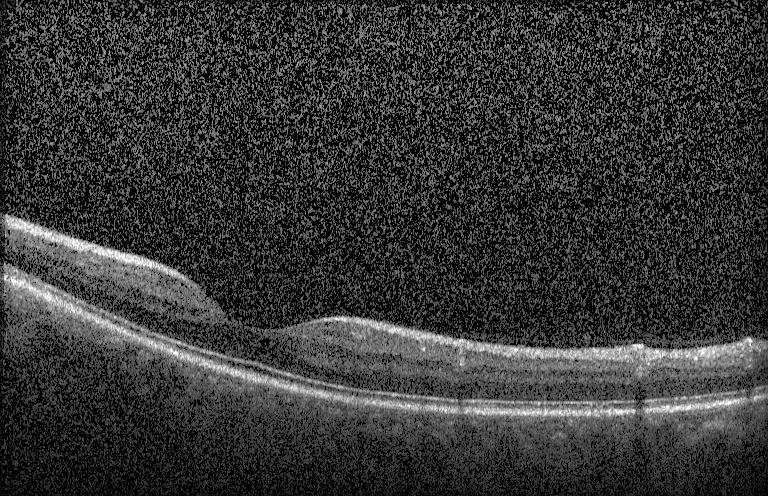

OCT line scan. Through the macula
No CNV, no DME, and no drusen.